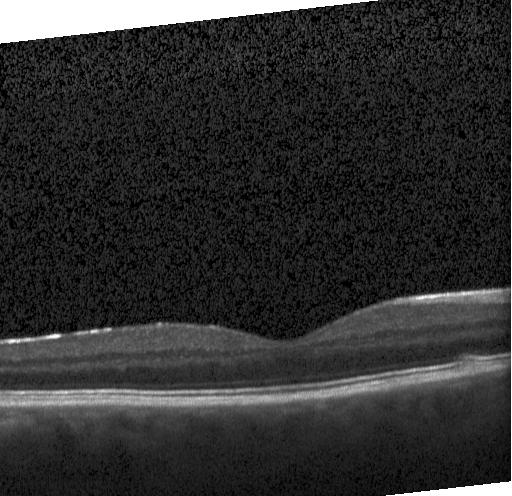

Assessment: drusen.